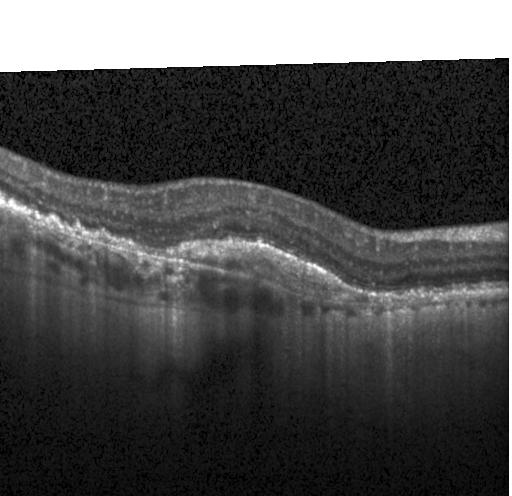
Dx: a choroidal neovascular membrane.